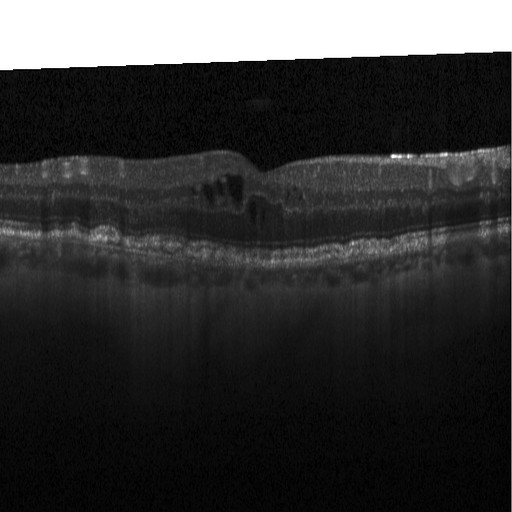

Finding: diabetic macular edema.